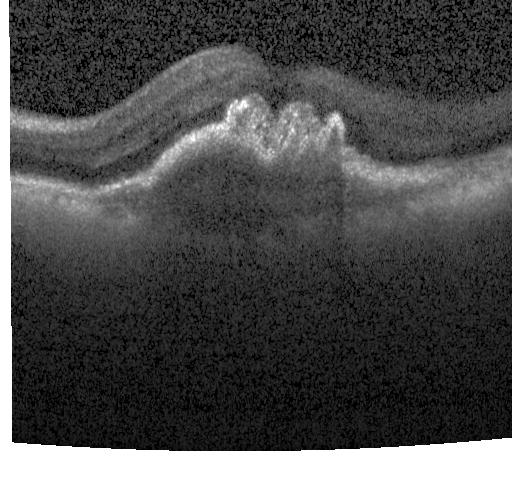
OCT line scan. Spectral-domain optical coherence tomography. The scan shows a choroidal neovascular membrane.